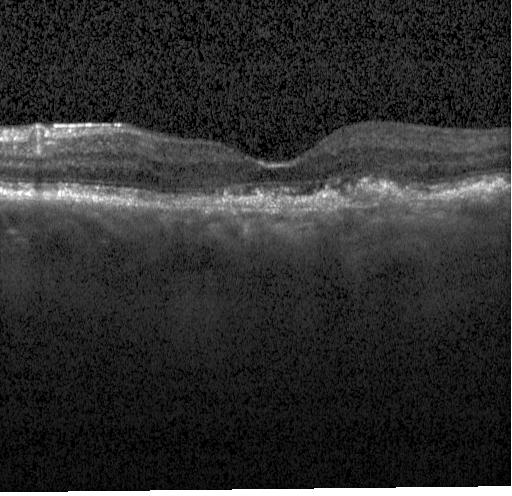

Retinal OCT cross-section
Diagnosis: choroidal neovascularization.